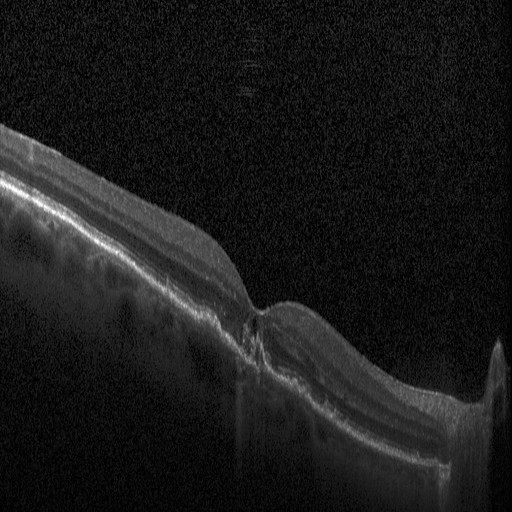

Impression: diabetic macular edema (DME).